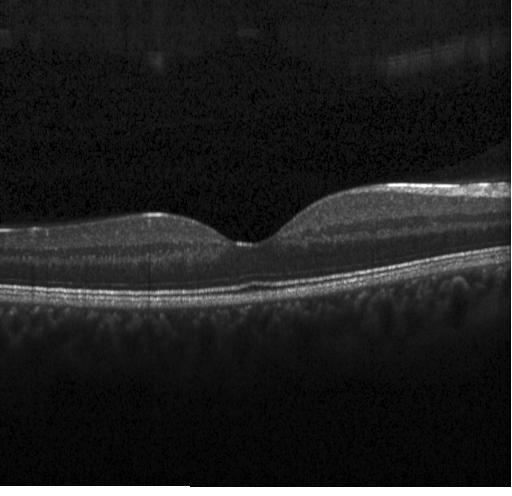 Spectral-domain OCT B-scan: no choroidal neovascularization, no diabetic macular edema, and no drusen.